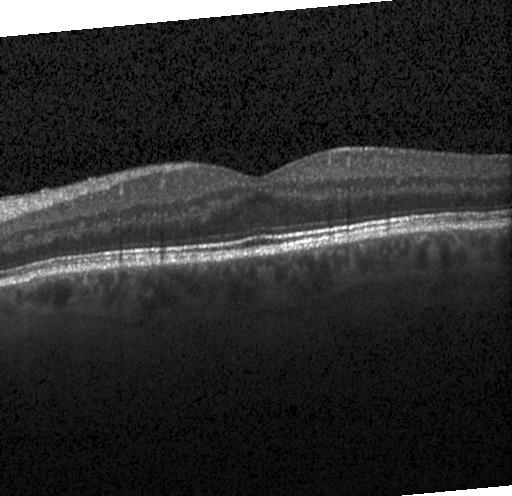
No choroidal neovascularization, no diabetic macular edema, and no drusen.